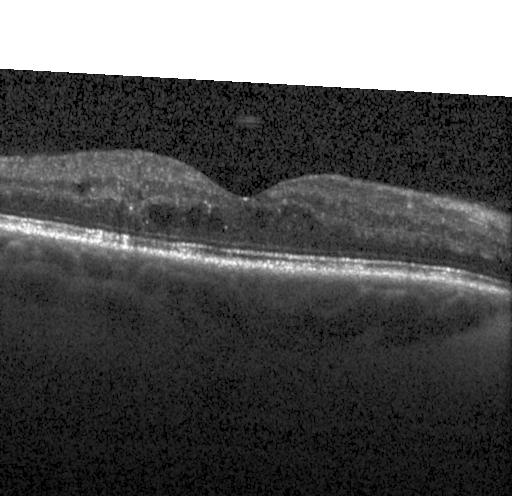
Instrument: Heidelberg Spectralis, OCT line scan, macular scan, SD-OCT. DME.